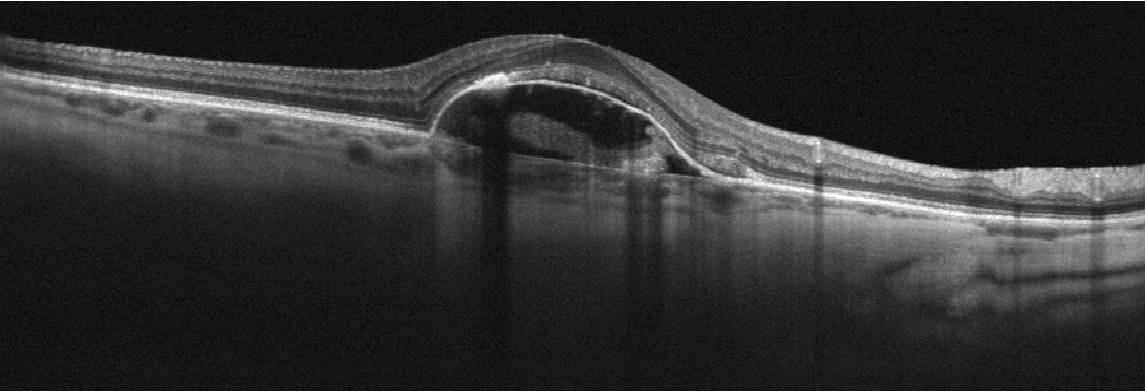 Optical coherence tomography B-scan; Optovue Avanti RTVue XR
Dx: age-related macular degeneration.